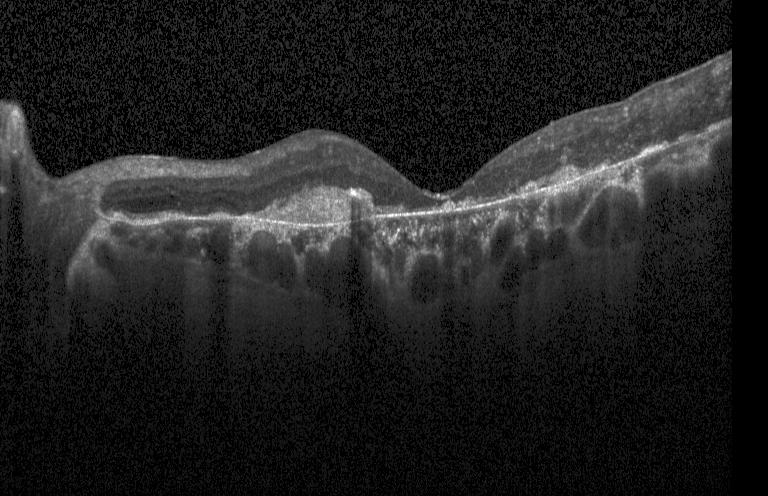

Finding: choroidal neovascularization (CNV).